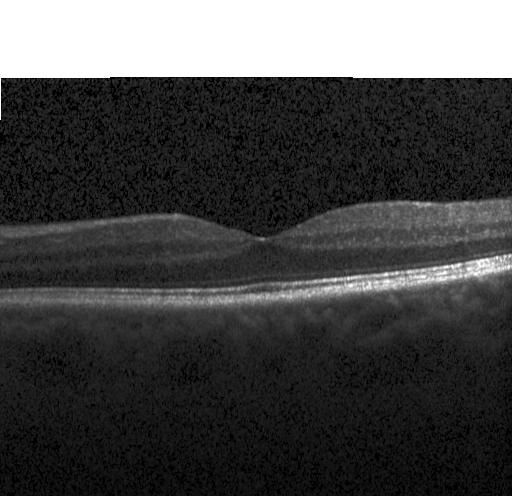
The scan shows no choroidal neovascularization, no diabetic macular edema, and no drusen.